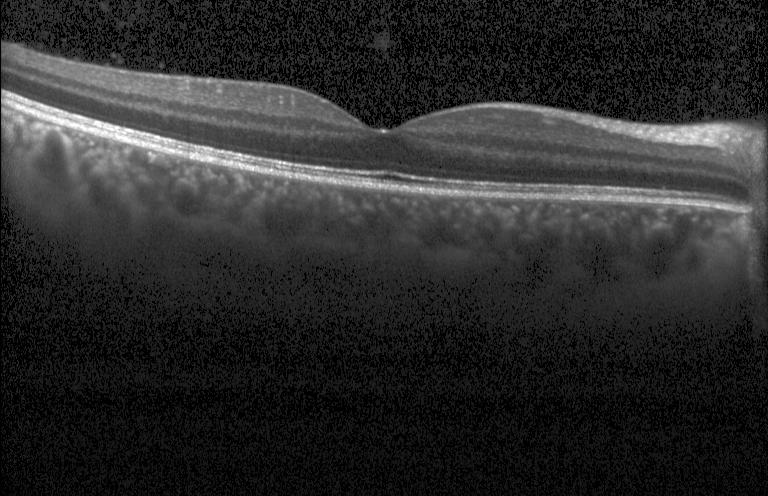
This B-scan demonstrates neither CNV, DME, nor drusen.